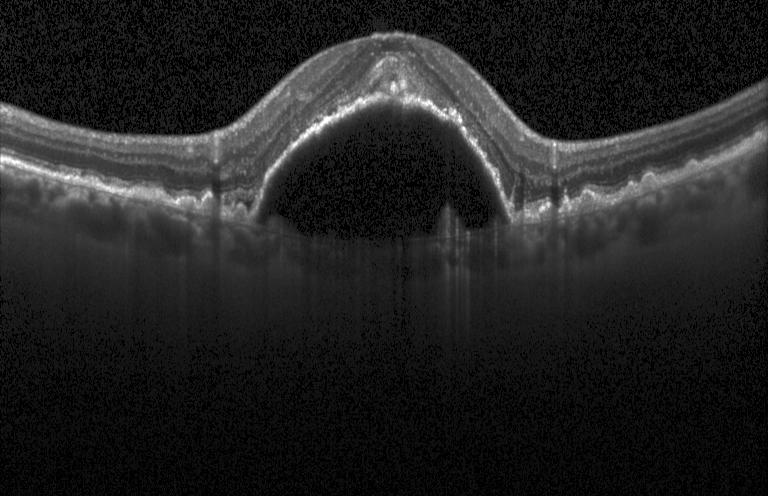 A choroidal neovascular membrane.